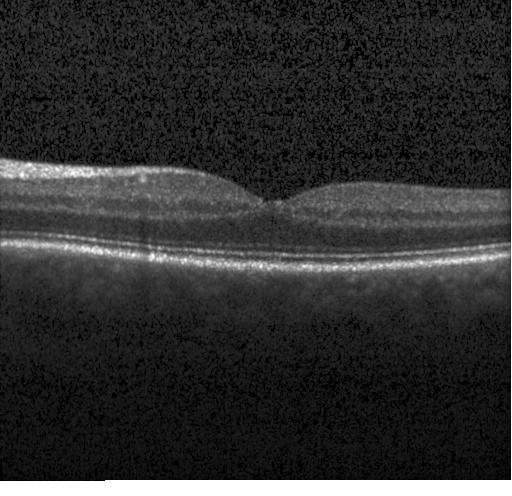 Retinal OCT cross-section. SD-OCT. Finding: no choroidal neovascularization, diabetic macular edema, or drusen.